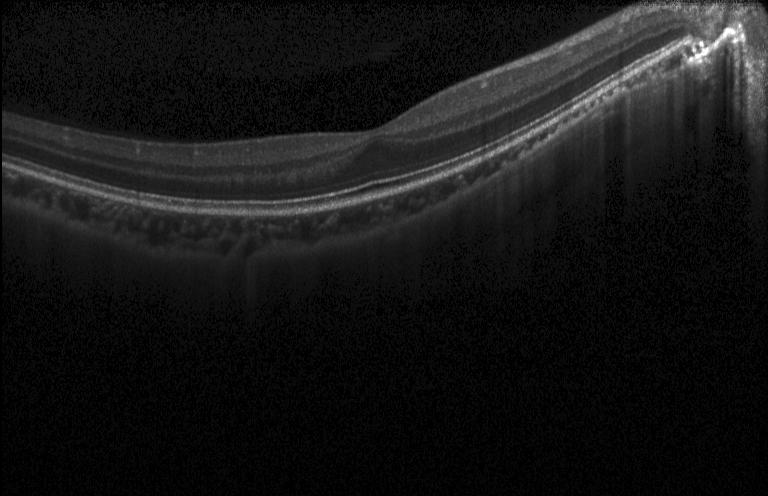 Spectral-domain optical coherence tomography; retinal OCT cross-section — Impression: no choroidal neovascularization, diabetic macular edema, or drusen.